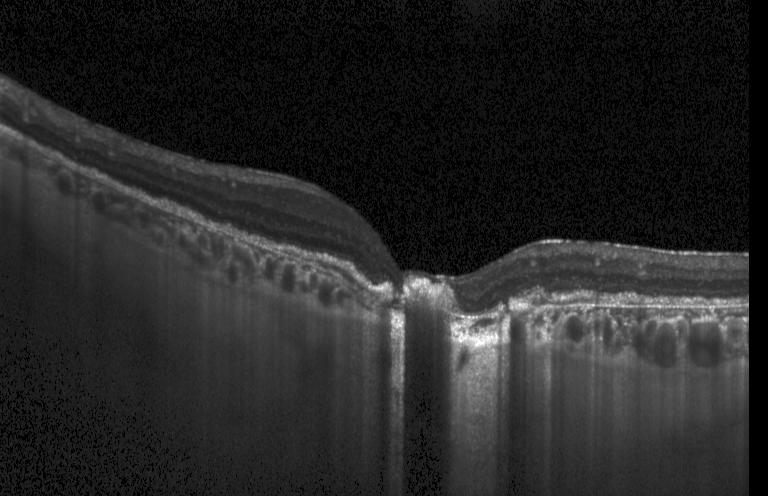
OCT finding: a choroidal neovascular membrane.